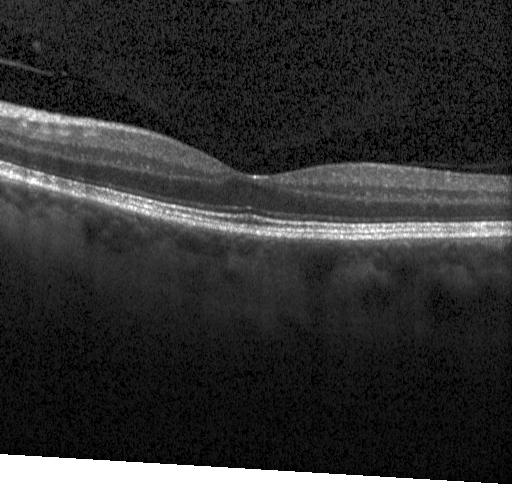
Heidelberg Spectralis · SD-OCT · retinal OCT cross-section · centered on the fovea
No evidence of CNV, DME, or drusen.